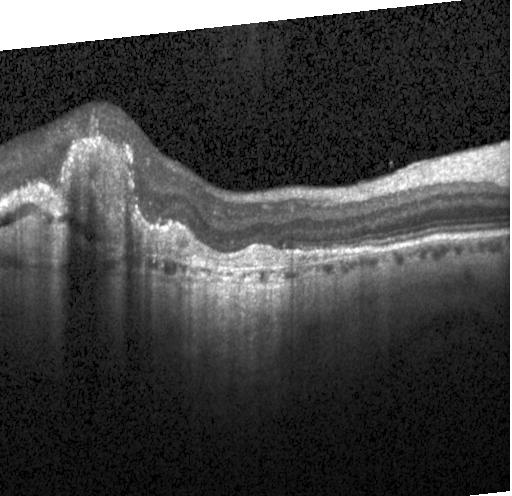
Retinal OCT cross-section showing CNV.